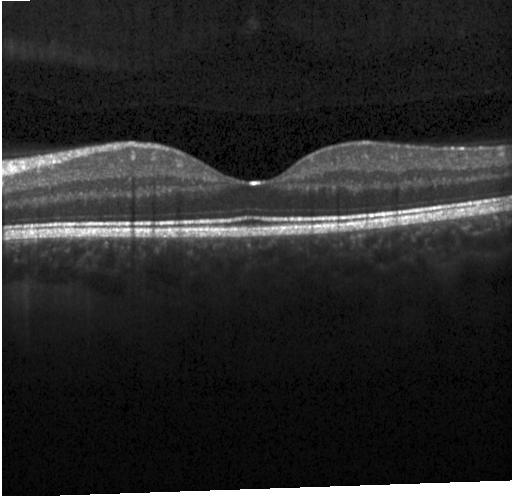
Macular OCT demonstrating neither choroidal neovascularization, diabetic macular edema, nor drusen.